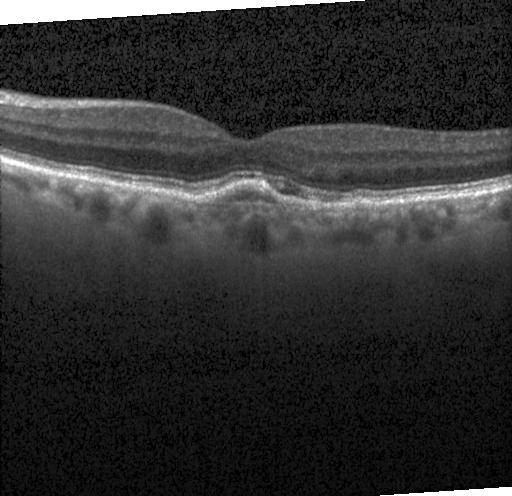
Fovea-centered; Heidelberg Spectralis; OCT line scan; SD-OCT. Finding: choroidal neovascularization.